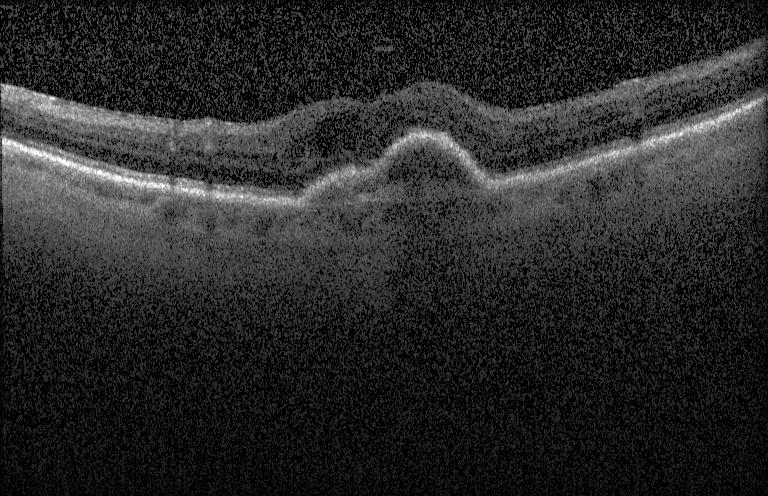

Retinal OCT cross-section. Heidelberg Spectralis OCT system. A choroidal neovascular membrane.